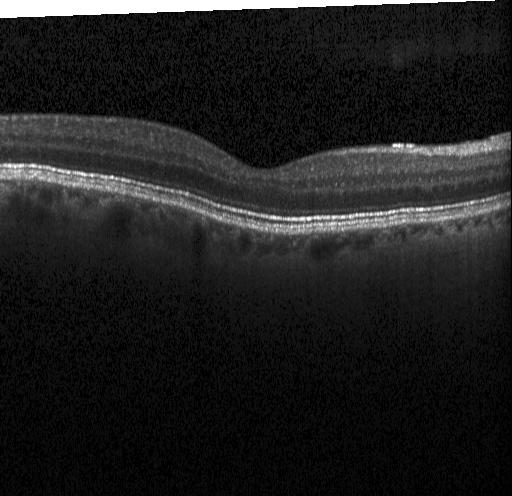
Fovea-centered. Optical coherence tomography scan. Acquired on a Heidelberg Spectralis. Spectral-domain OCT
OCT finding: no CNV, DME, or drusen.